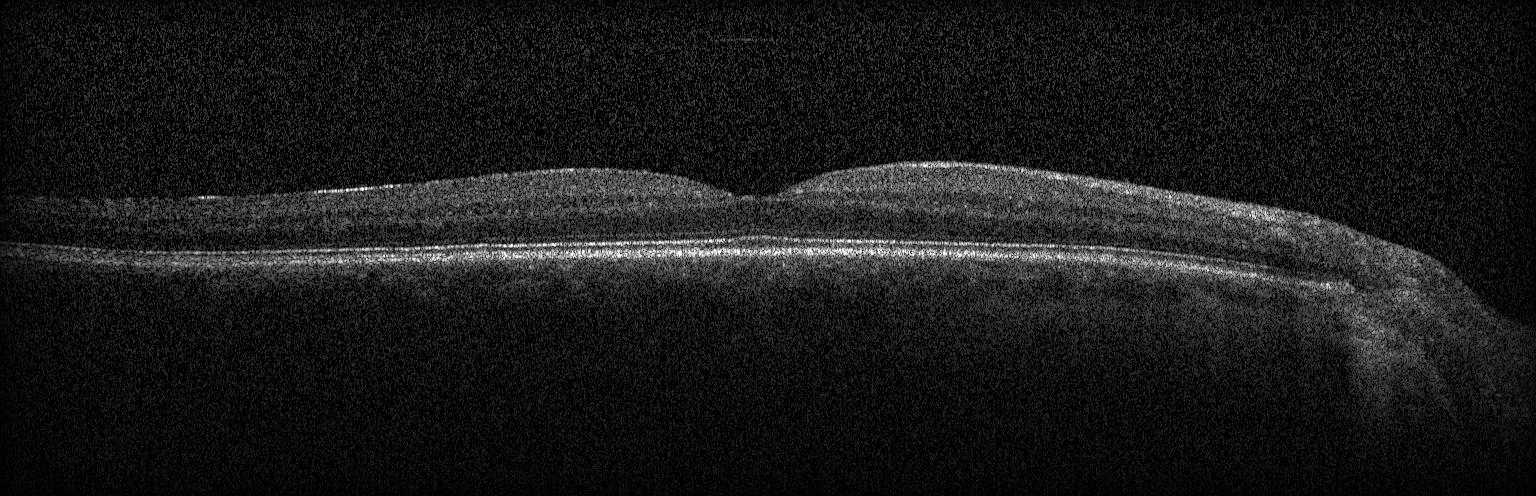

Optical coherence tomography B-scan — Assessment: neither CNV, DME, nor drusen.